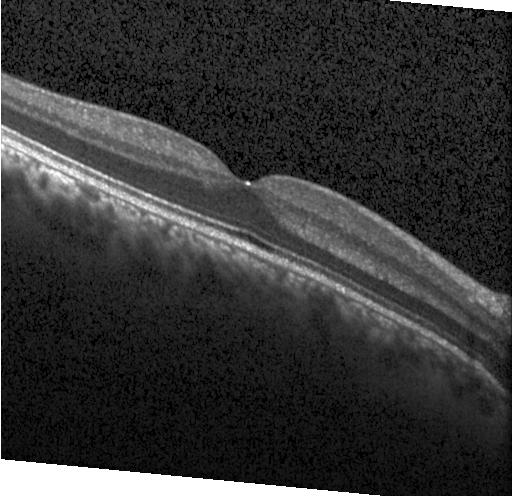
Retinal OCT cross-section. The scan shows no CNV, DME, or drusen.